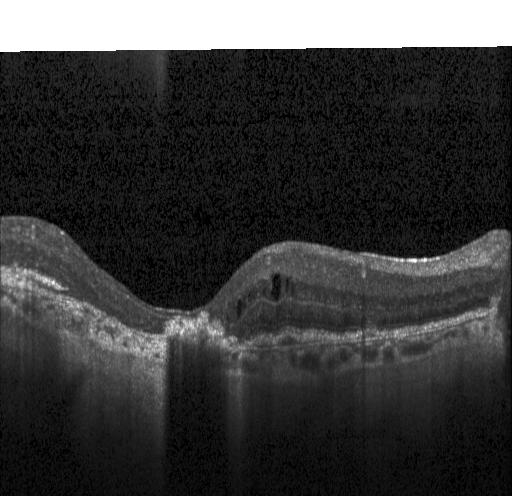

OCT scan showing choroidal neovascularization.